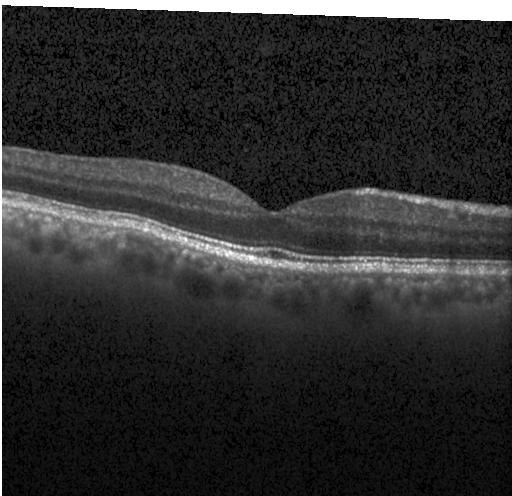

Assessment: no choroidal neovascularization, no diabetic macular edema, and no drusen.